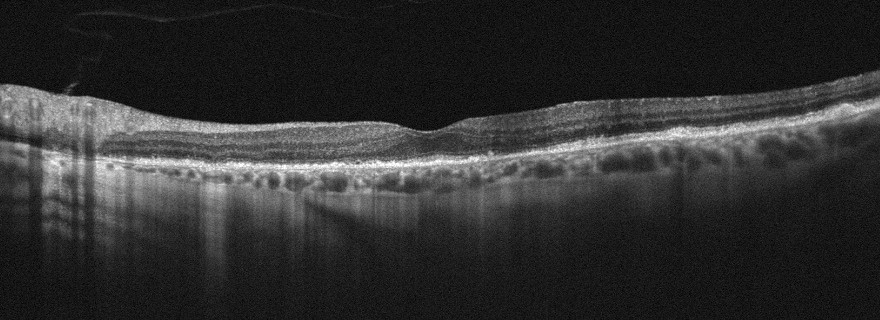 OCT B-scan · acquired on an Optovue Avanti RTVue XR · fovea-centered.
Dx: age-related macular degeneration.